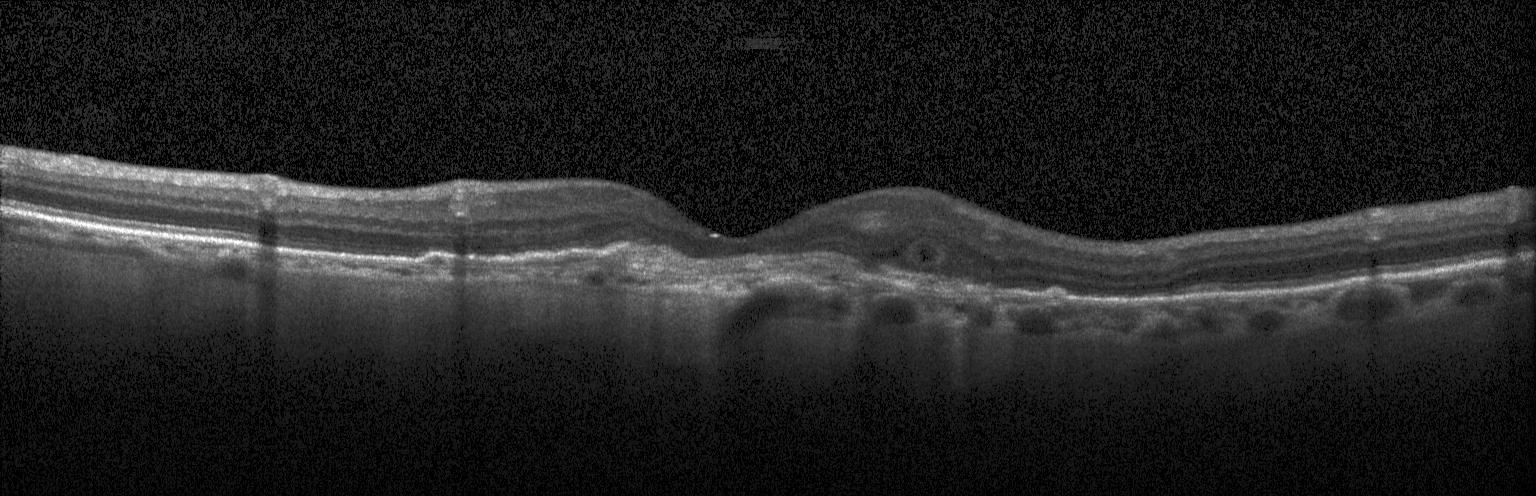

Impression: choroidal neovascularization.